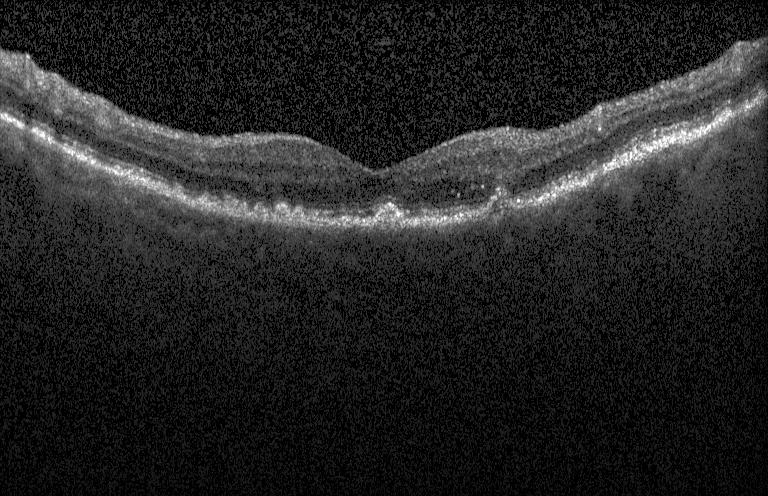

Diagnosis: a choroidal neovascular membrane.